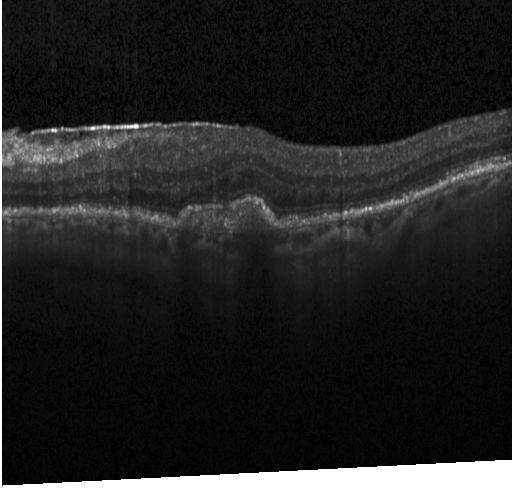
Spectral-domain optical coherence tomography; centered on the fovea; Heidelberg Spectralis OCT system; retinal OCT cross-section — Finding: a choroidal neovascular membrane.